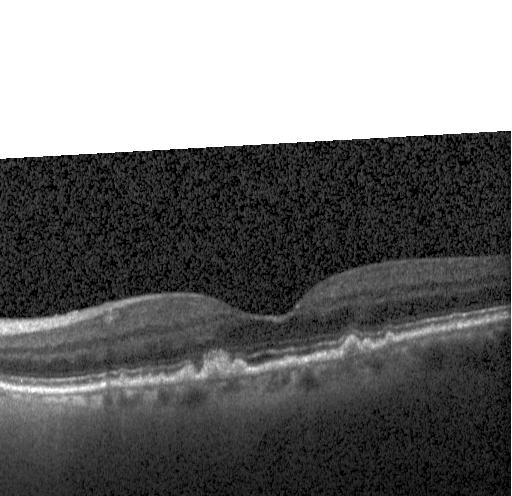 OCT B-scan
Dx: sub-RPE drusenoid deposits.